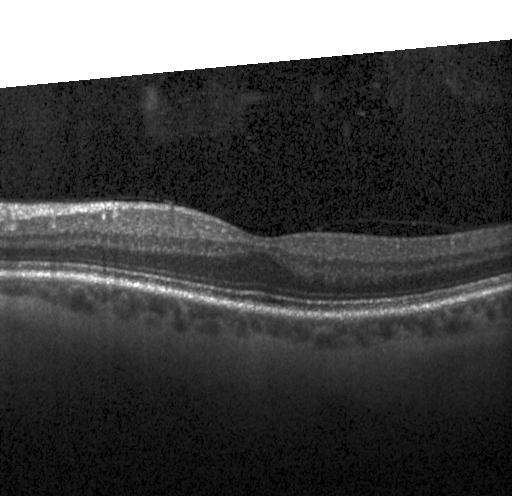

Heidelberg Spectralis · spectral-domain OCT · OCT B-scan
No choroidal neovascularization, no diabetic macular edema, and no drusen.